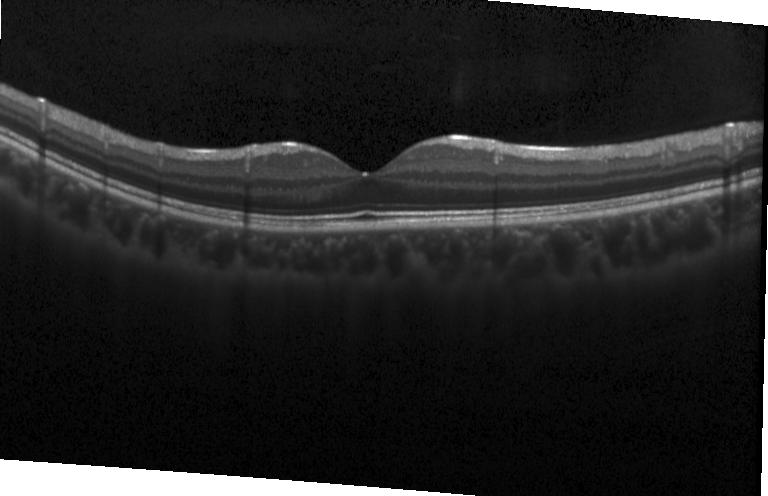 No choroidal neovascularization, no diabetic macular edema, and no drusen.